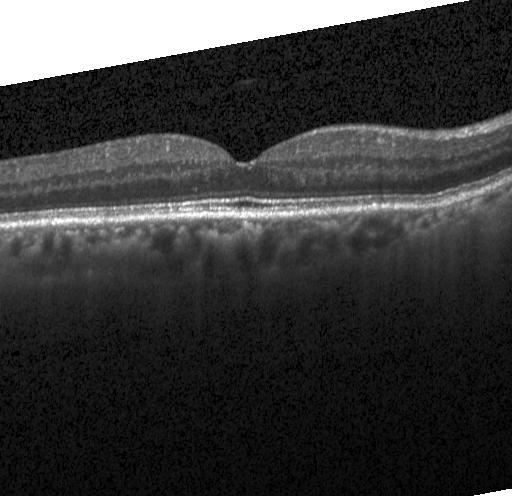 Retinal OCT cross-section. Assessment: no choroidal neovascularization, diabetic macular edema, or drusen.